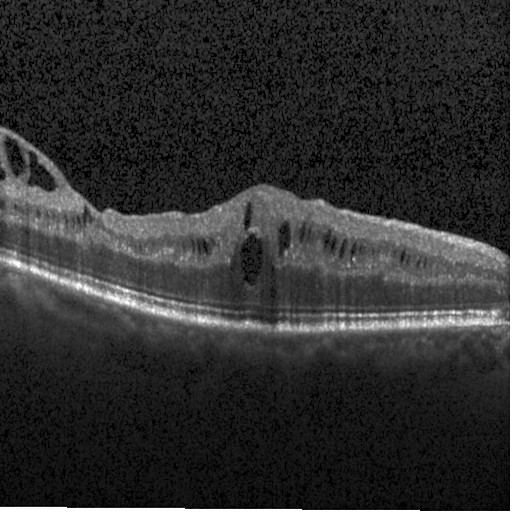
Macular OCT: DME.